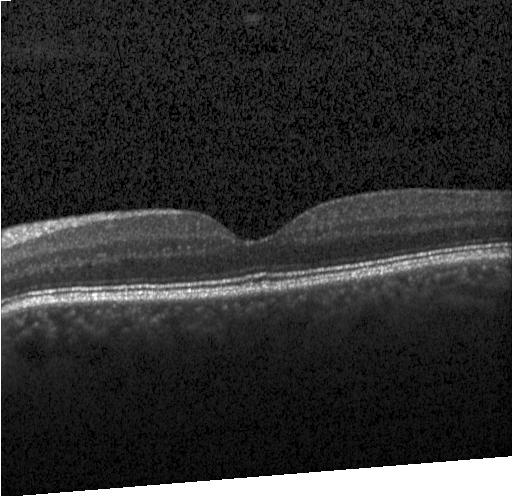

Optical coherence tomography B-scan — Finding: no choroidal neovascularization, diabetic macular edema, or drusen.